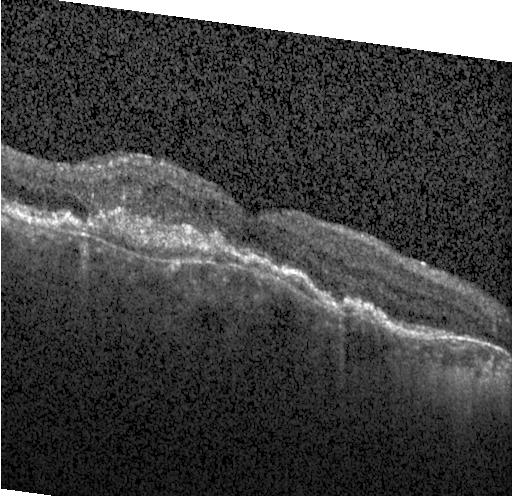

Retinal OCT B-scan.
Diagnosis: a choroidal neovascular membrane.